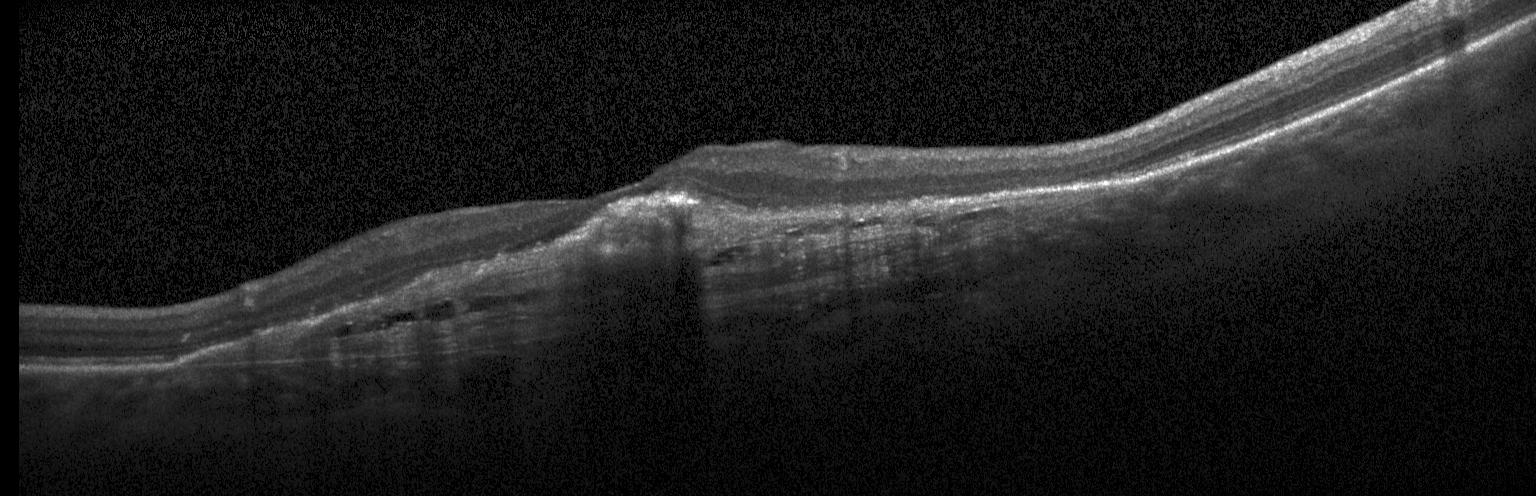 Retinal OCT B-scan. SD-OCT
Assessment: CNV.